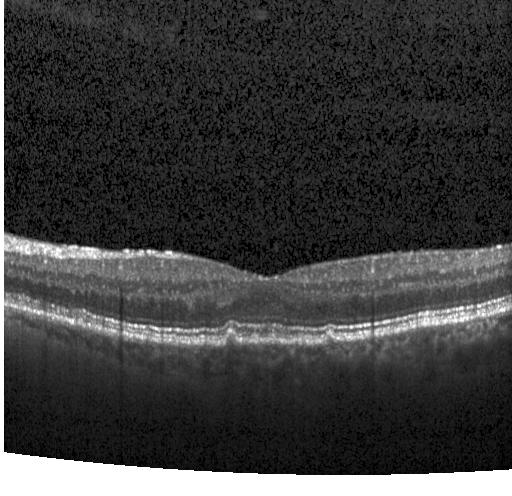

Finding: drusen.